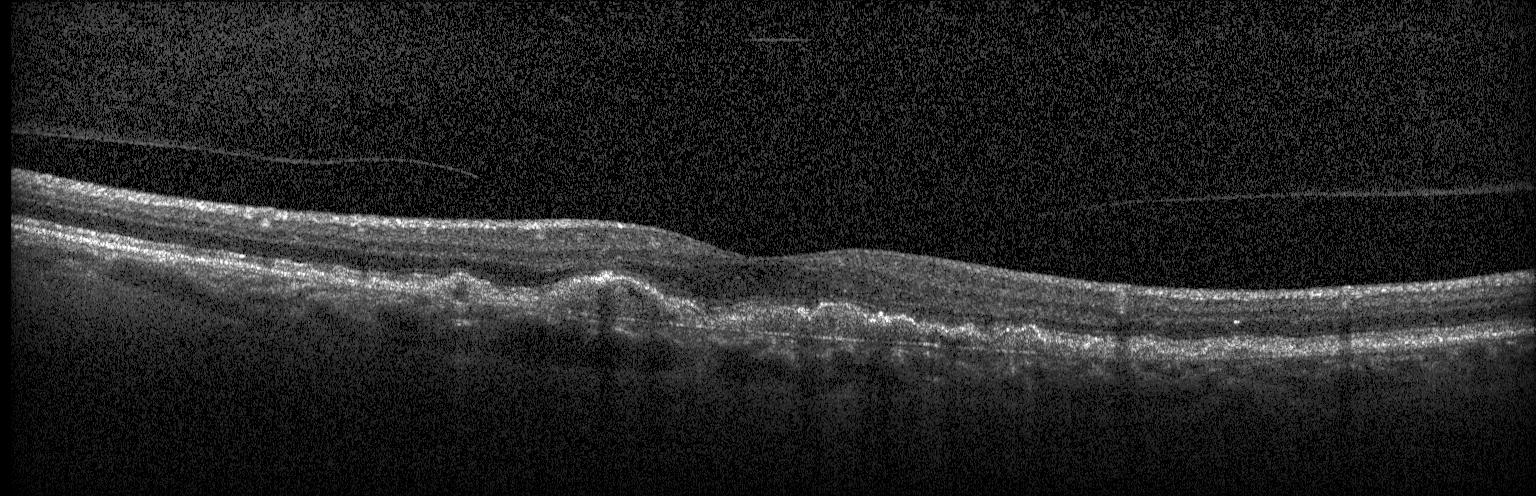 SD-OCT, Heidelberg Spectralis OCT system, retinal OCT cross-section
Impression: a choroidal neovascular membrane.